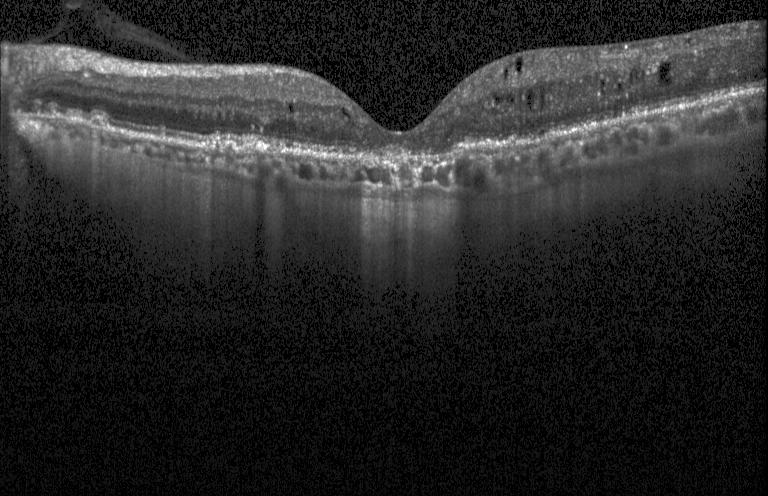 Optical coherence tomography B-scan, SD-OCT, through the macula. OCT finding: choroidal neovascularization.